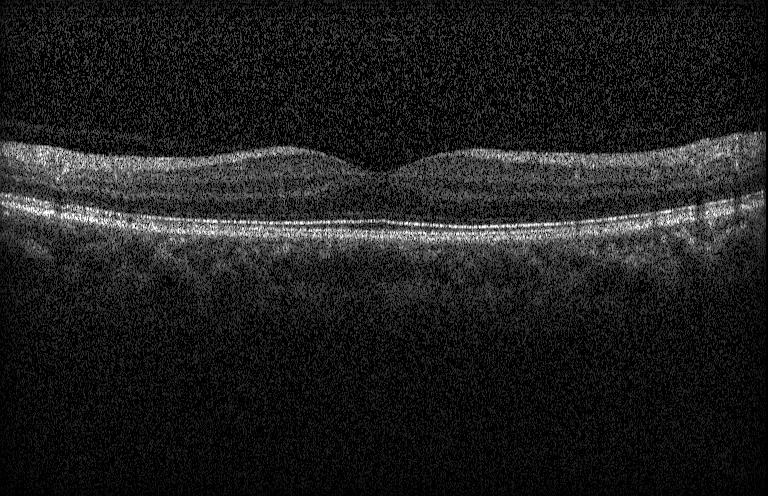
OCT B-scan. Spectral-domain OCT. Instrument: Heidelberg Spectralis. Centered on the fovea — Diagnosis: no evidence of CNV, DME, or drusen.